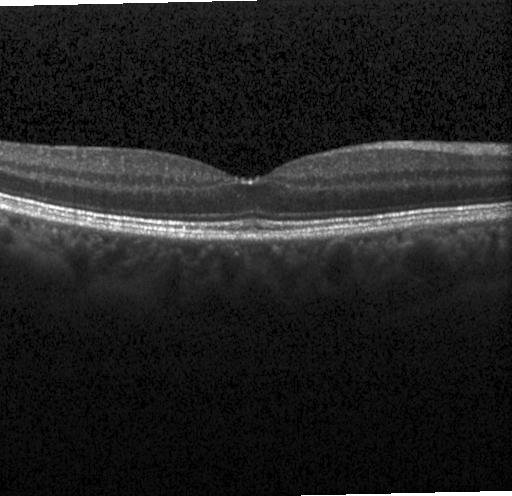

OCT scan showing no evidence of choroidal neovascularization, diabetic macular edema, or drusen.